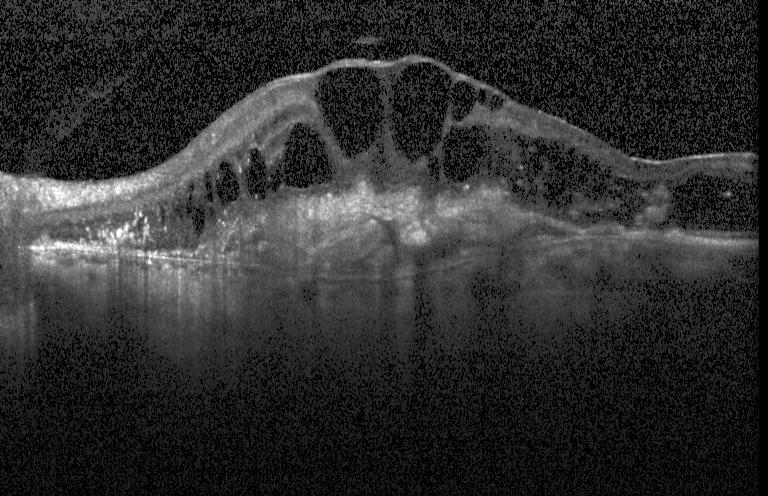

Retinal OCT cross-section.
Macular OCT: choroidal neovascularization (CNV).